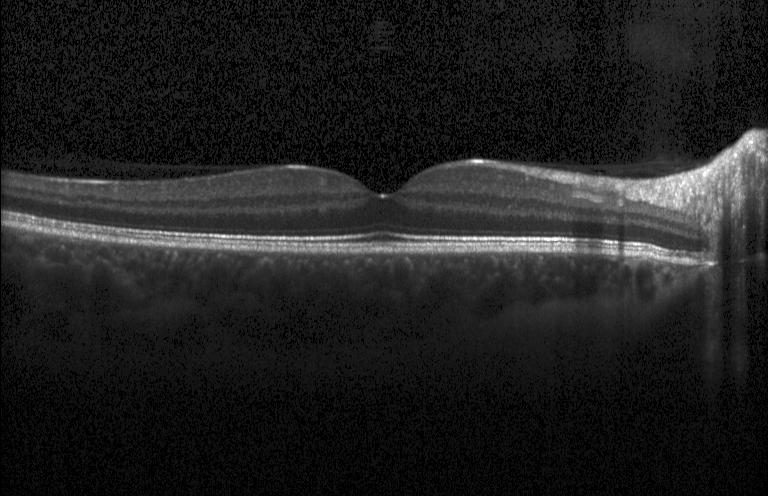

Retinal OCT B-scan. Diagnosis: no CNV, DME, or drusen.